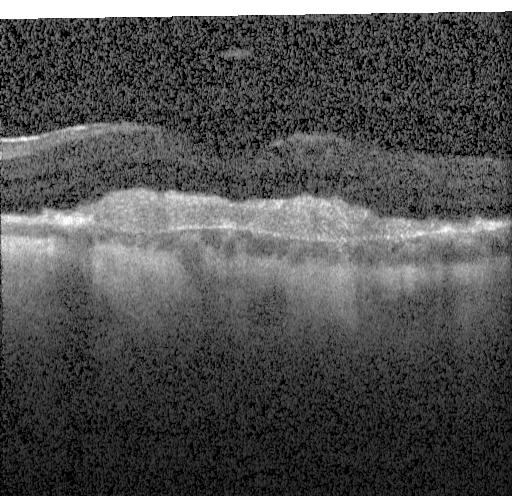
OCT line scan.
This B-scan demonstrates a choroidal neovascular membrane.